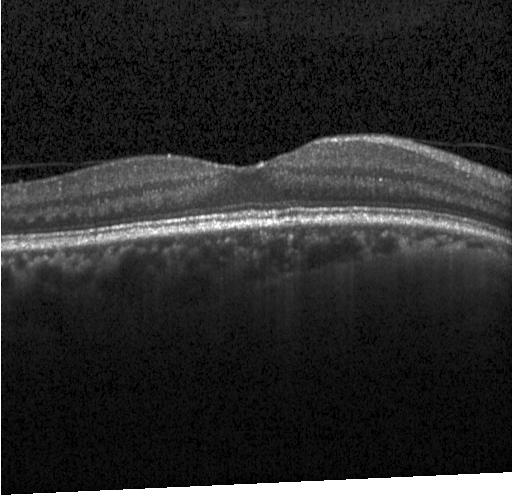 Optical coherence tomography scan · centered on the fovea. Assessment: no evidence of choroidal neovascularization, diabetic macular edema, or drusen.